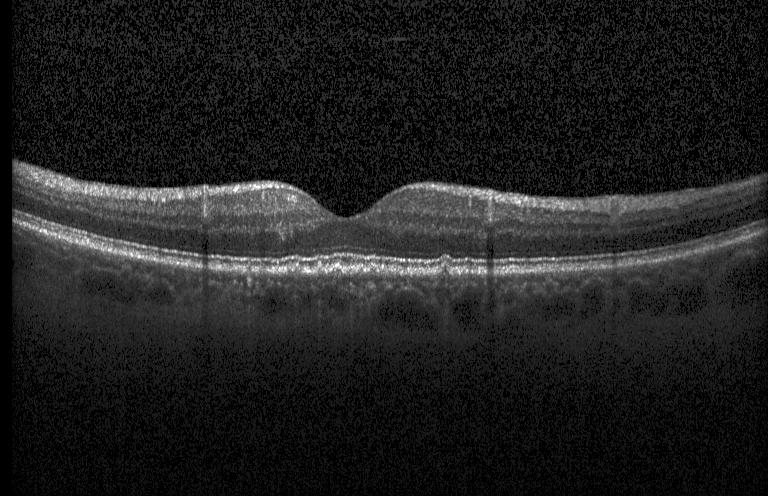
Finding: sub-RPE drusenoid deposits.